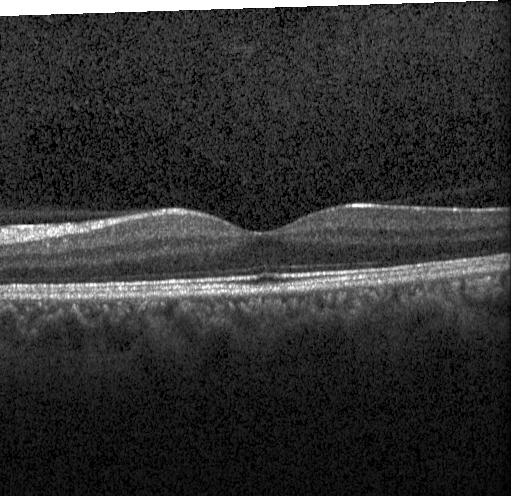
Optical coherence tomography scan
Diagnosis: neither choroidal neovascularization, diabetic macular edema, nor drusen.